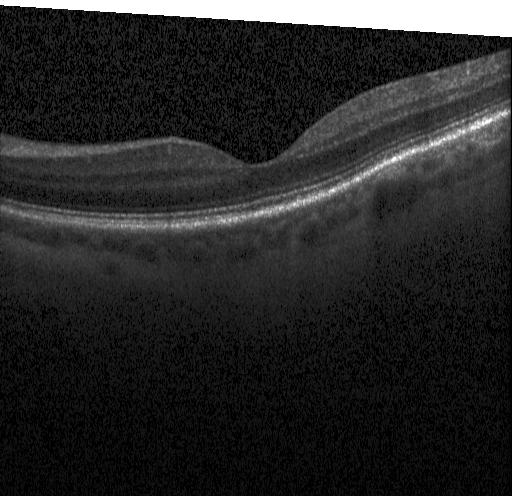

Finding: neither choroidal neovascularization, diabetic macular edema, nor drusen.